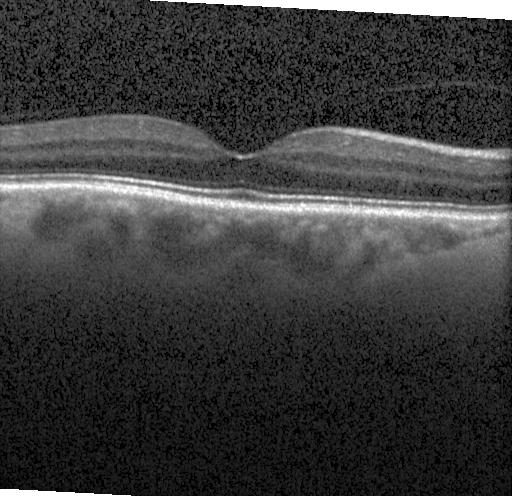 Through the macula, retinal OCT cross-section. Assessment: no evidence of choroidal neovascularization, diabetic macular edema, or drusen.